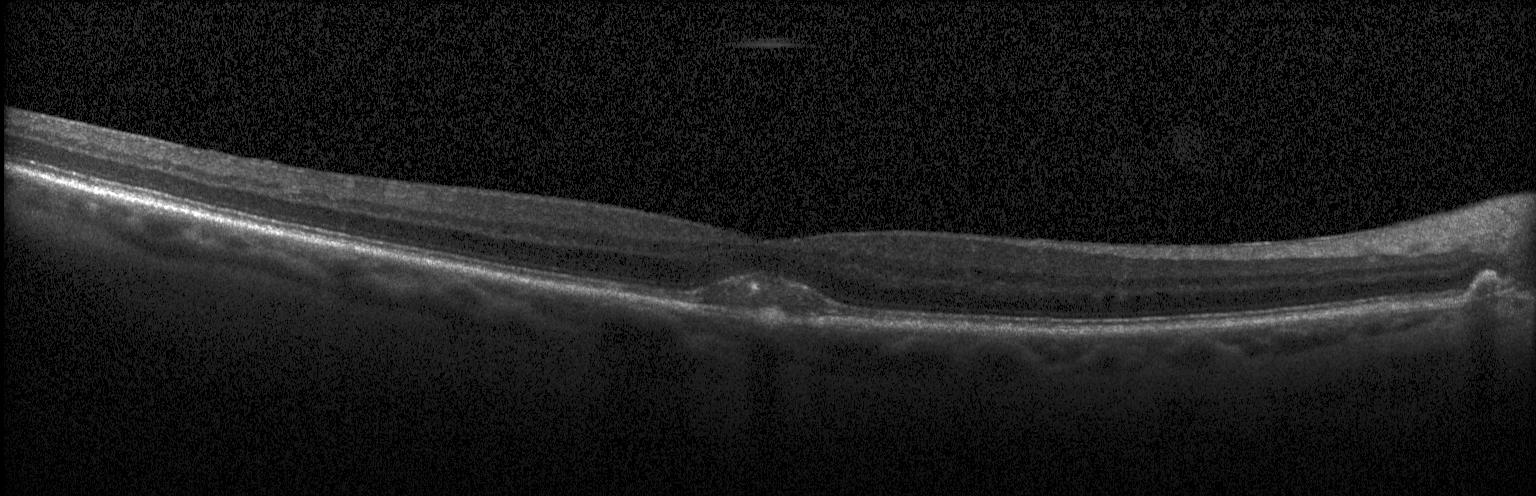

Optical coherence tomography scan — Impression: a choroidal neovascular membrane.